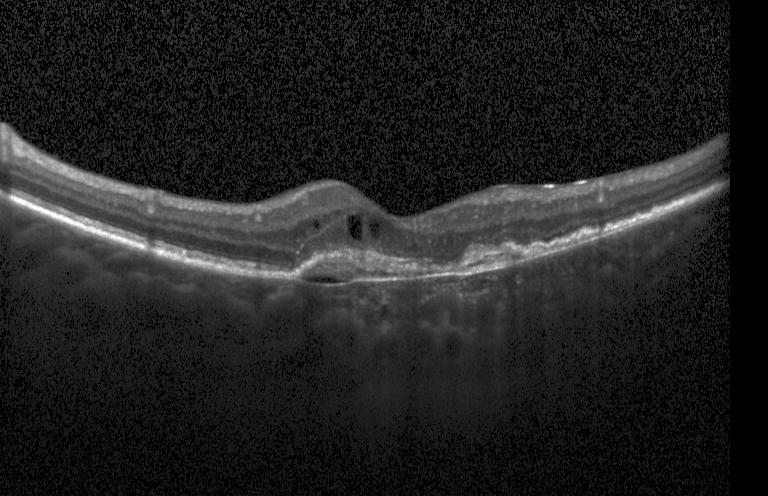 Retinal OCT B-scan; spectral-domain optical coherence tomography; horizontal scan through the fovea — Diagnosis: a choroidal neovascular membrane.